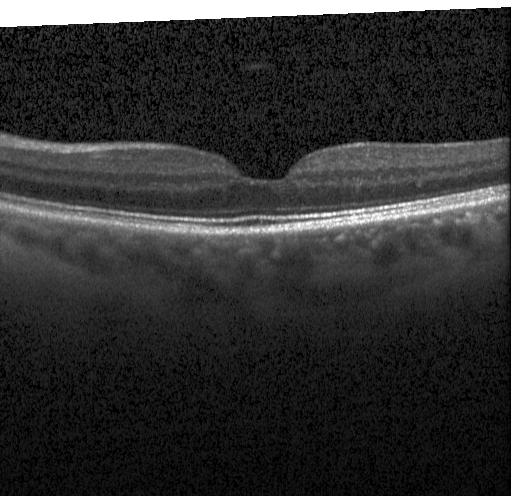 Instrument: Heidelberg Spectralis · spectral-domain OCT · retinal OCT B-scan
Assessment: no choroidal neovascularization, no diabetic macular edema, and no drusen.